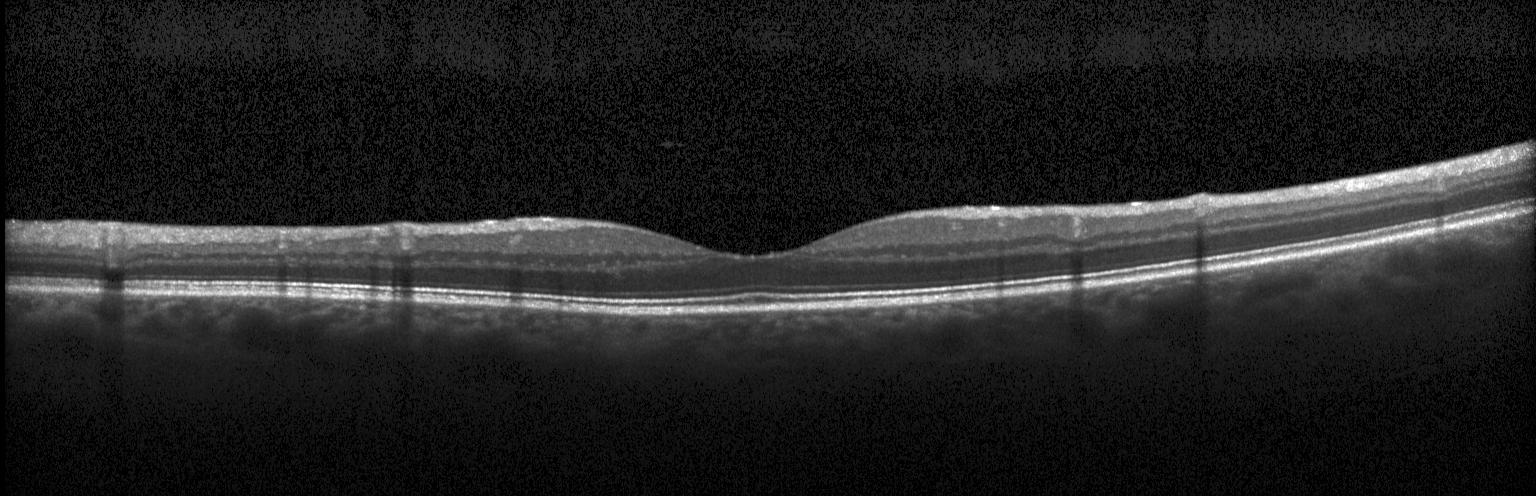

Macular scan · optical coherence tomography scan.
Diagnosis: no choroidal neovascularization, diabetic macular edema, or drusen.